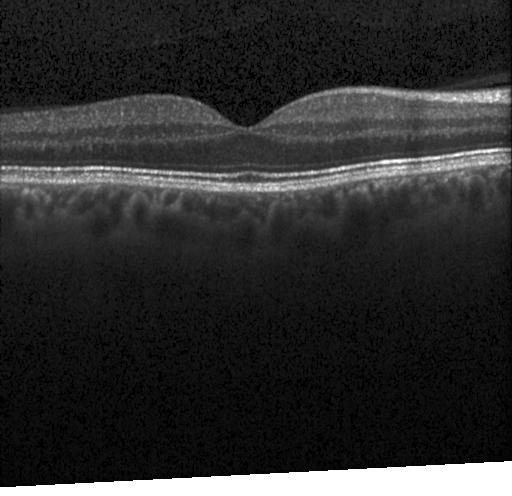 Acquired on a Heidelberg Spectralis. OCT line scan. SD-OCT. Through the macula.
Diagnosis: neither choroidal neovascularization, diabetic macular edema, nor drusen.